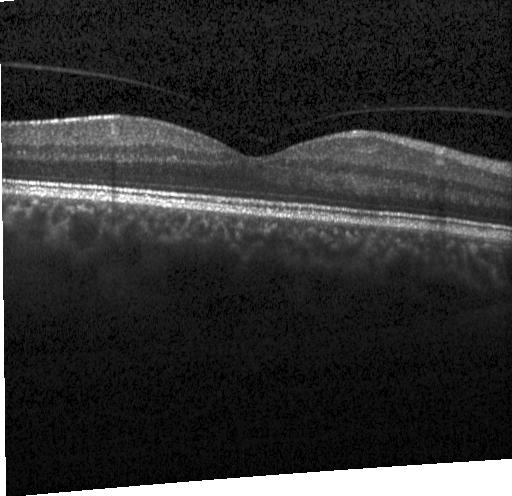 OCT B-scan
No choroidal neovascularization, no diabetic macular edema, and no drusen.